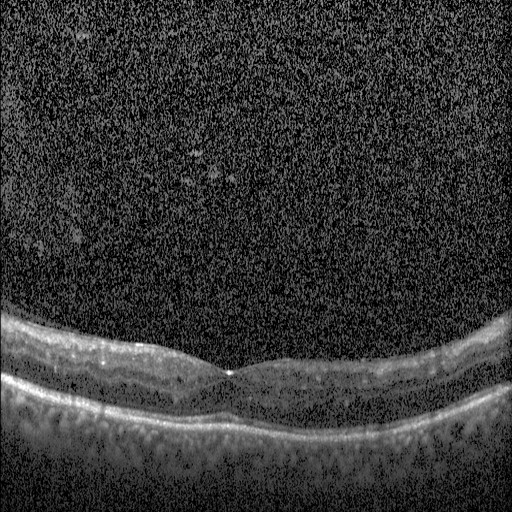

Diagnosis: diabetic macular edema.